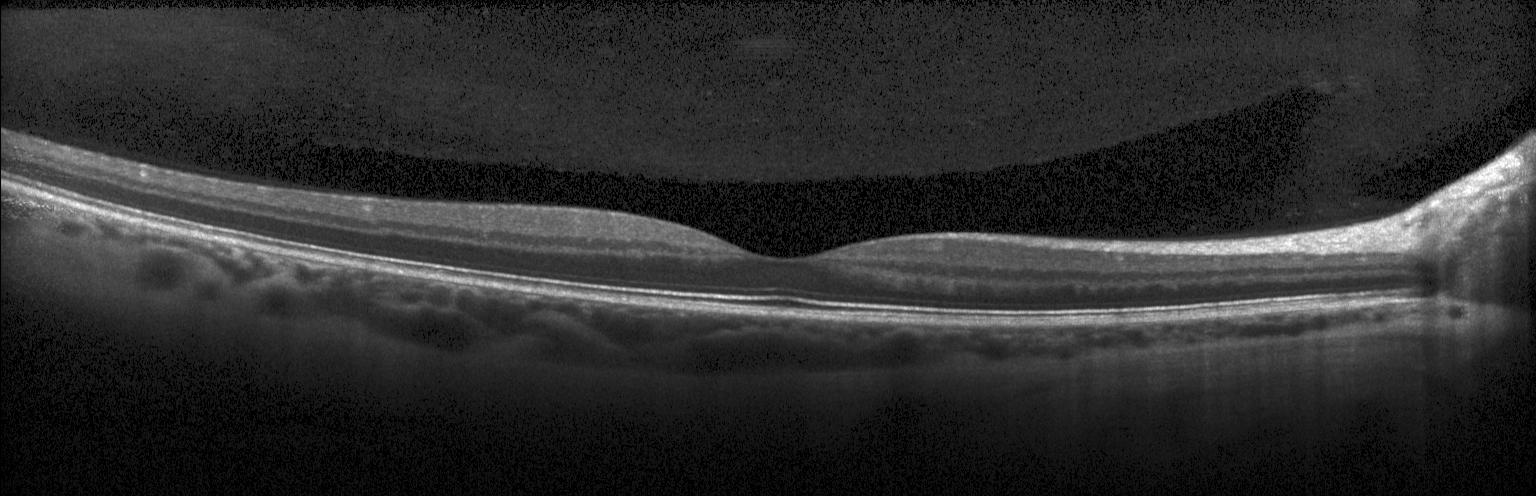 Optical coherence tomography B-scan; acquired on a Heidelberg Spectralis — OCT finding: neither choroidal neovascularization, diabetic macular edema, nor drusen.